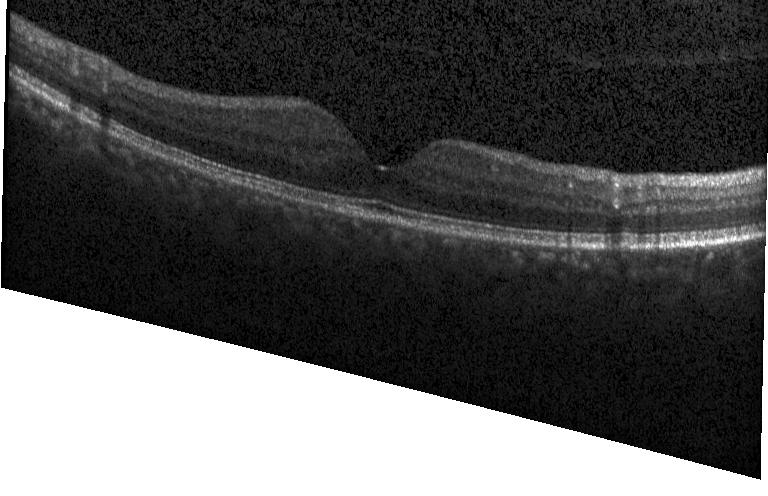
Optical coherence tomography scan — Finding: no choroidal neovascularization, diabetic macular edema, or drusen.